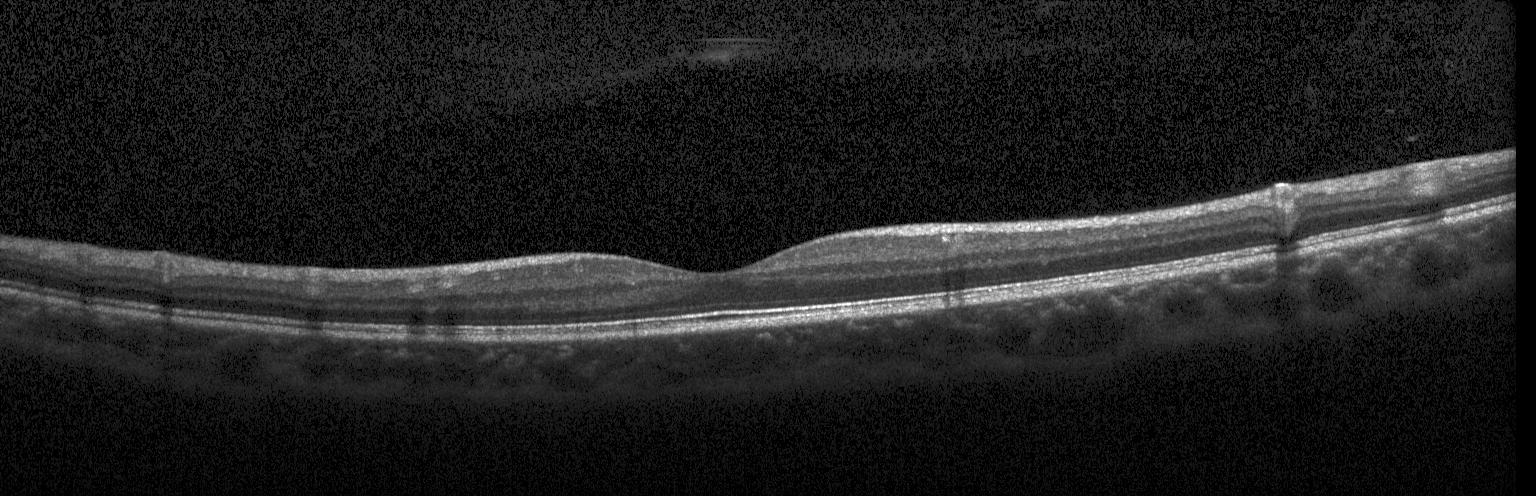
Impression: no CNV, DME, or drusen.